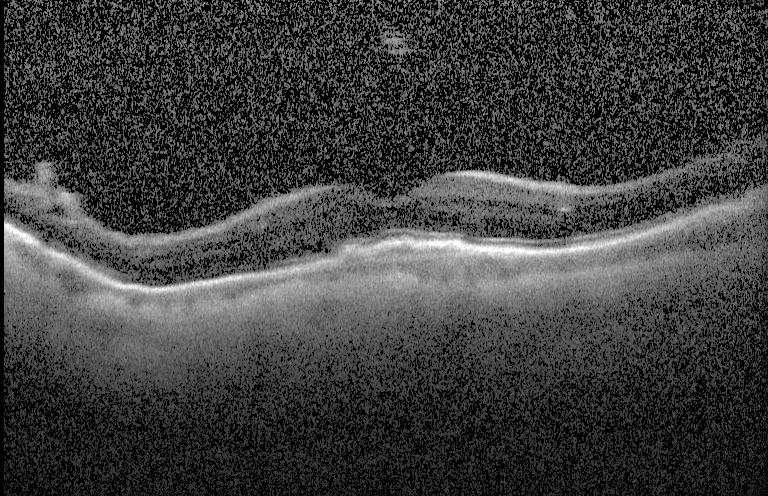

Diagnosis: choroidal neovascularization (CNV).